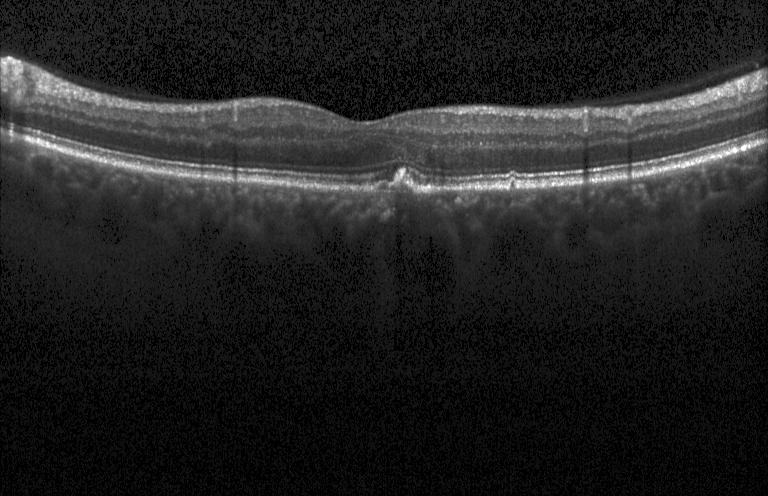
Optical coherence tomography scan; spectral-domain OCT.
Diagnosis: drusen.